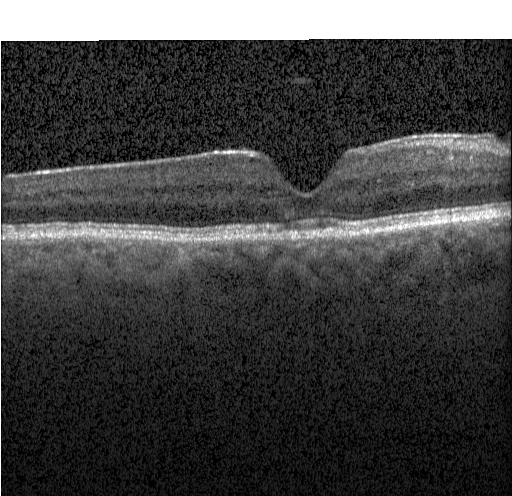
SD-OCT. Fovea-centered. Heidelberg Spectralis OCT system. OCT B-scan
Impression: no CNV, no DME, and no drusen.